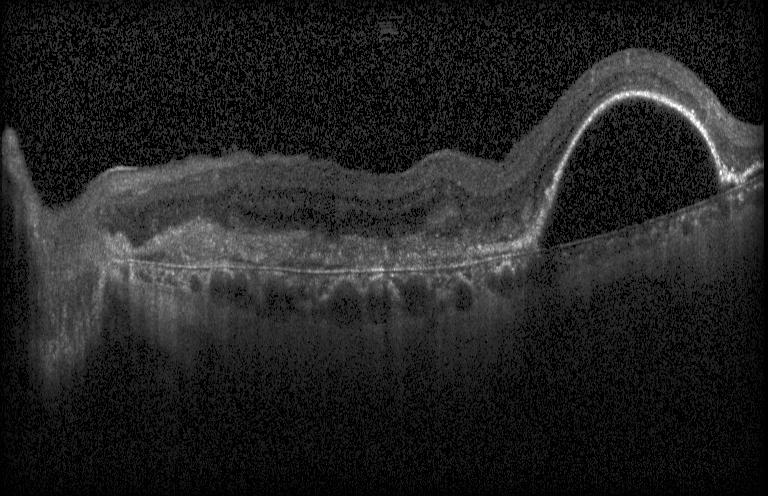 Fovea-centered; retinal OCT B-scan; spectral-domain optical coherence tomography — Diagnosis: choroidal neovascularization (CNV).